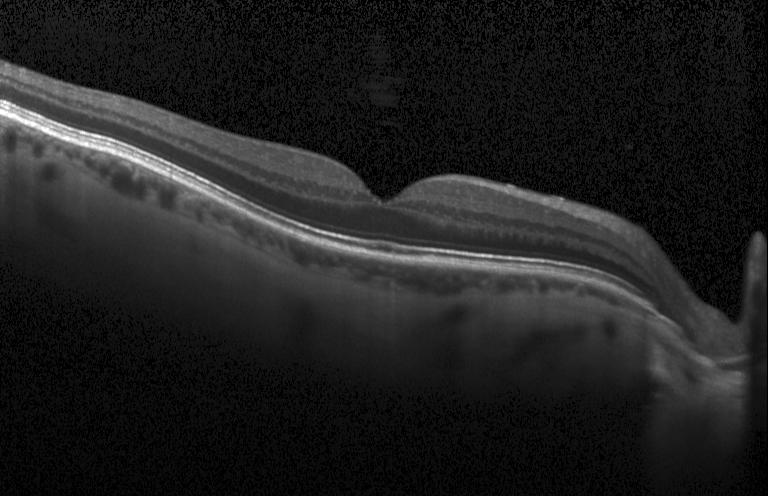
OCT line scan
Impression: no choroidal neovascularization, diabetic macular edema, or drusen.